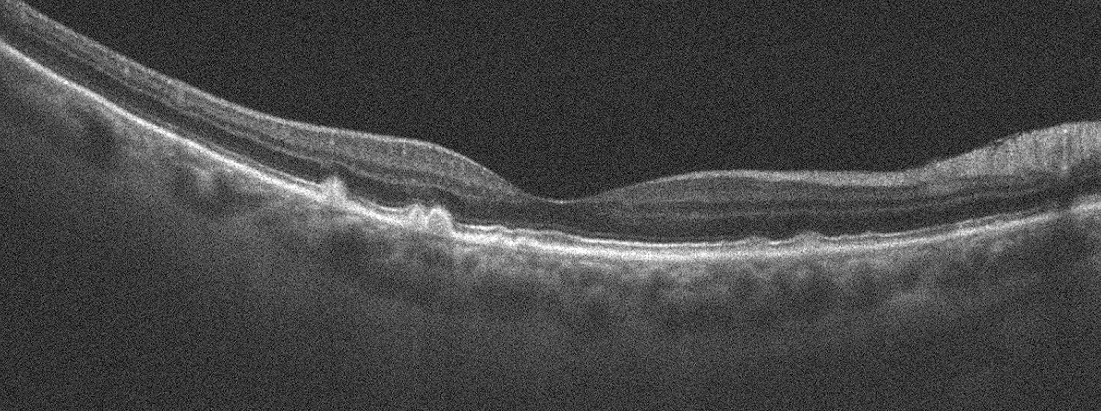 OCT scan showing AMD.